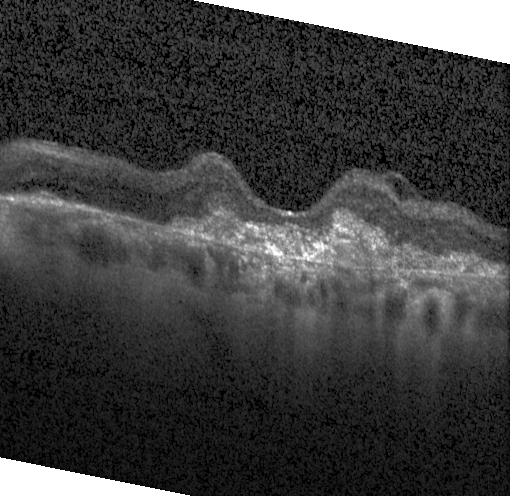
Assessment: a choroidal neovascular membrane.